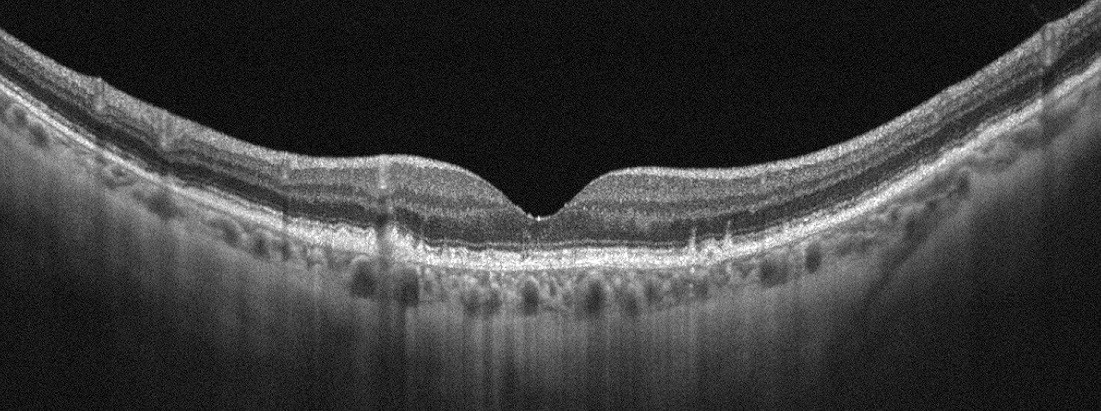 Through the macula. Retinal OCT B-scan. Optovue Avanti RTVue XR
The scan shows AMD.